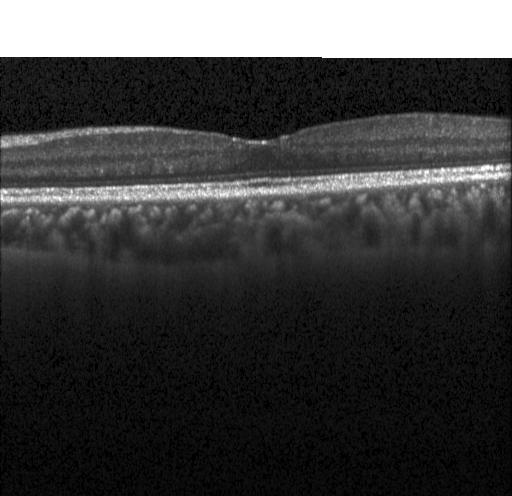

Fovea-centered, spectral-domain optical coherence tomography, optical coherence tomography B-scan. Finding: neither choroidal neovascularization, diabetic macular edema, nor drusen.